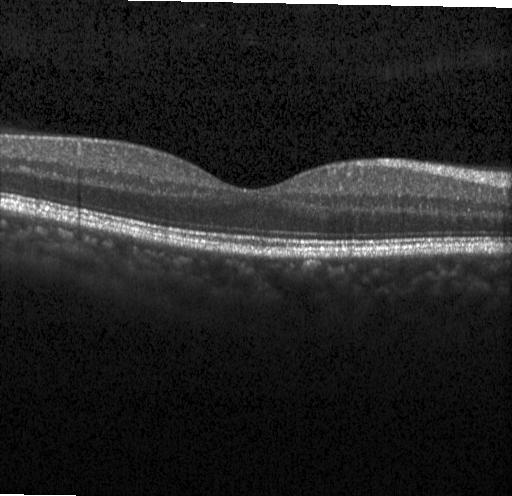 The scan shows no CNV, no DME, and no drusen.